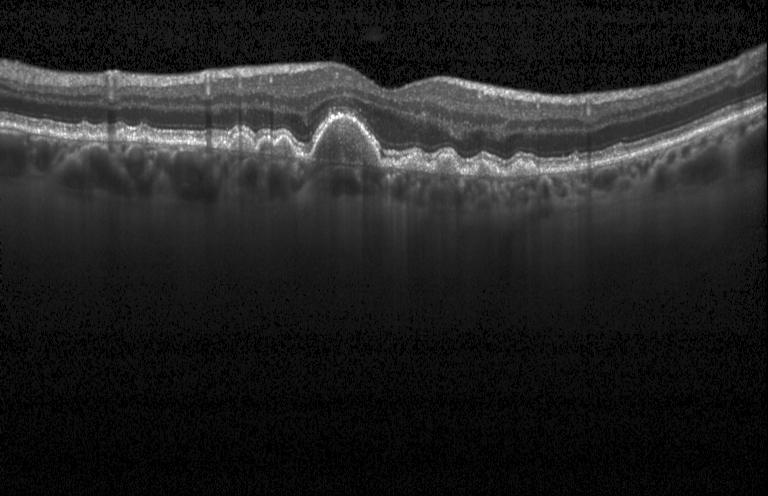
Diagnosis: sub-RPE drusenoid deposits.